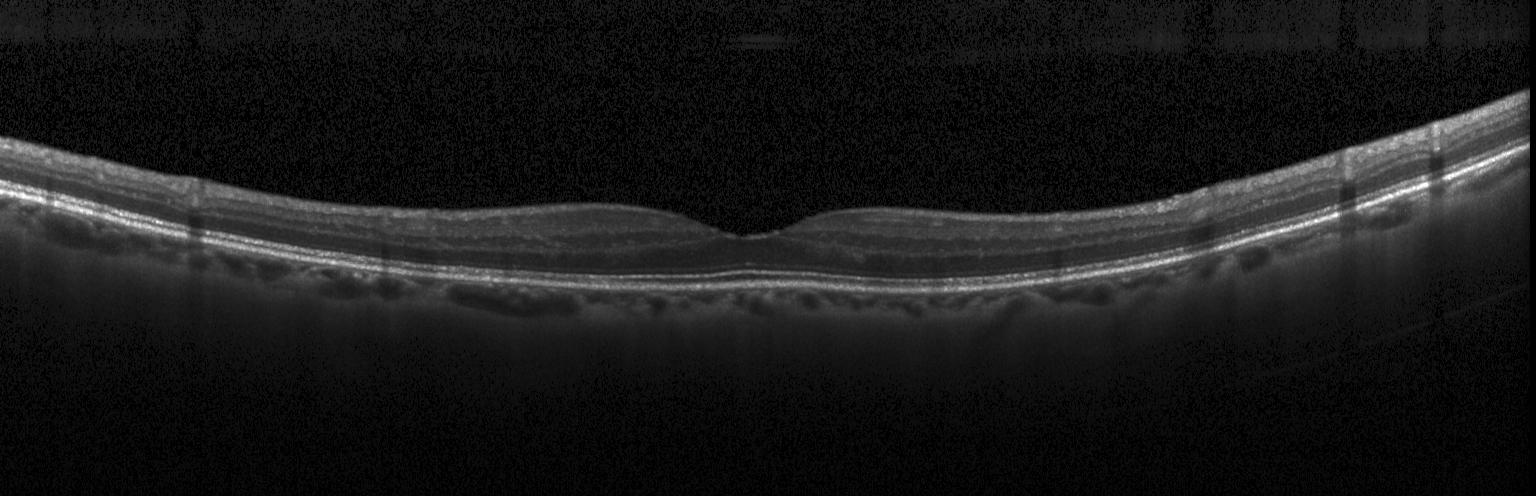
OCT line scan, fovea-centered, SD-OCT — Impression: no choroidal neovascularization, no diabetic macular edema, and no drusen.